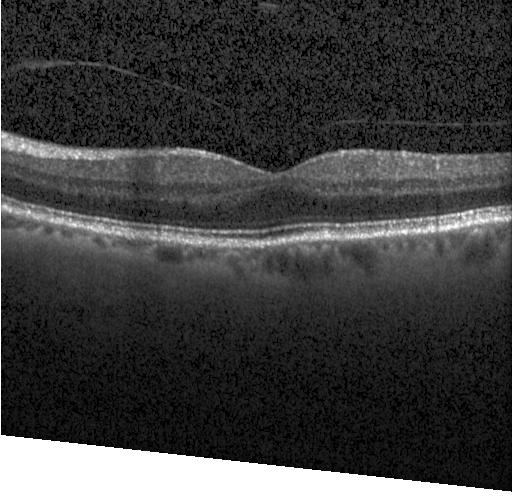 Finding: neither choroidal neovascularization, diabetic macular edema, nor drusen.